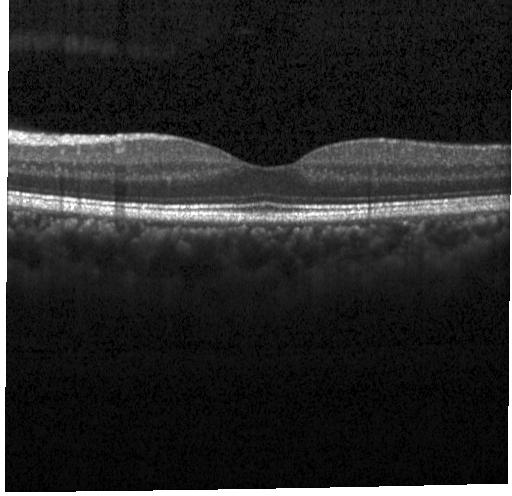

Instrument: Heidelberg Spectralis · OCT B-scan. Dx: neither choroidal neovascularization, diabetic macular edema, nor drusen.